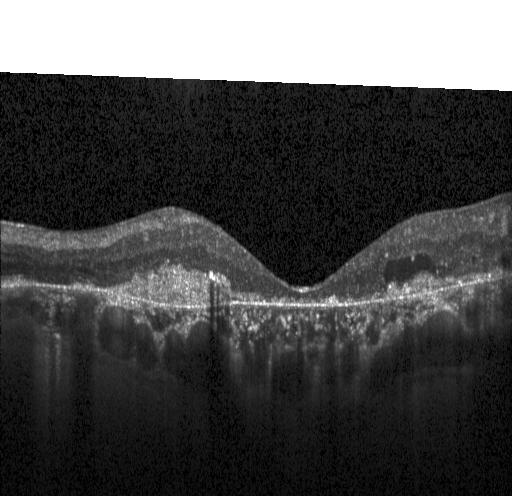

Finding: choroidal neovascularization (CNV).